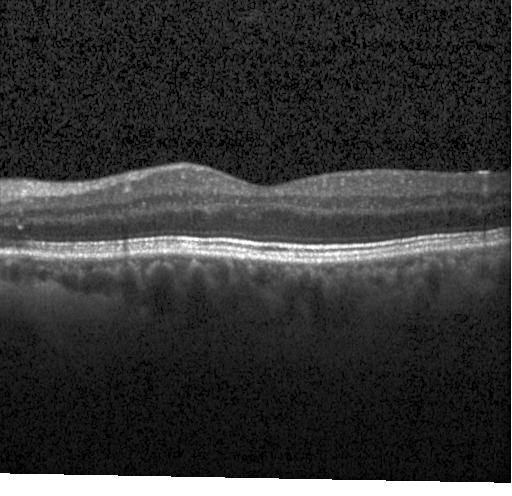 OCT line scan. Instrument: Heidelberg Spectralis.
The scan shows no choroidal neovascularization, diabetic macular edema, or drusen.